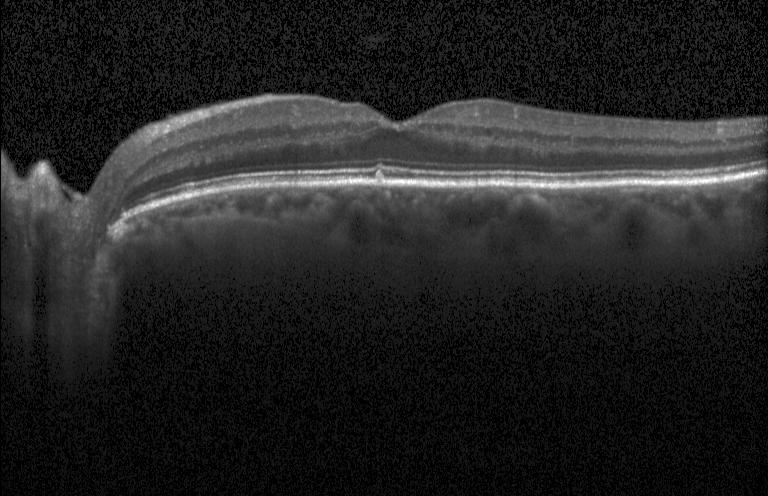 Instrument: Heidelberg Spectralis · OCT line scan · spectral-domain OCT — Impression: drusen.